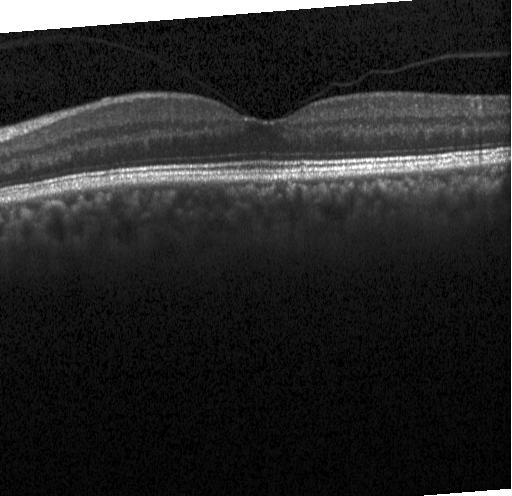

OCT B-scan, macular scan
Assessment: neither choroidal neovascularization, diabetic macular edema, nor drusen.